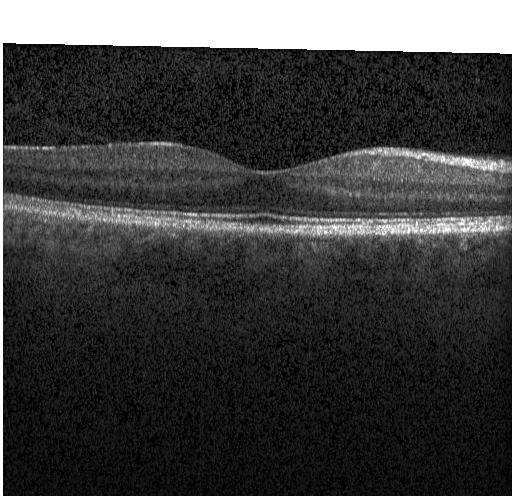
Retinal OCT B-scan; instrument: Heidelberg Spectralis; SD-OCT. Dx: no evidence of choroidal neovascularization, diabetic macular edema, or drusen.